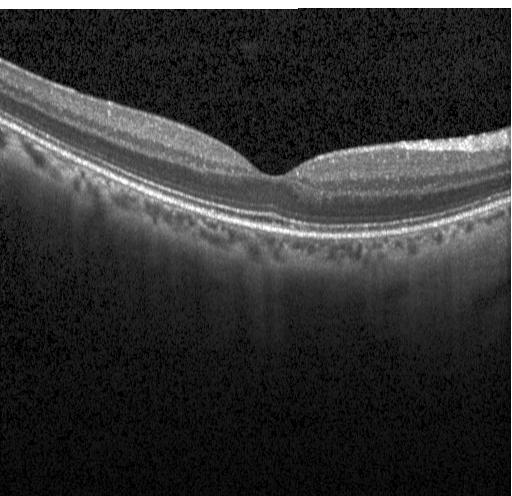 Centered on the fovea. Acquired on a Heidelberg Spectralis. OCT line scan. Spectral-domain OCT
Finding: no choroidal neovascularization, no diabetic macular edema, and no drusen.